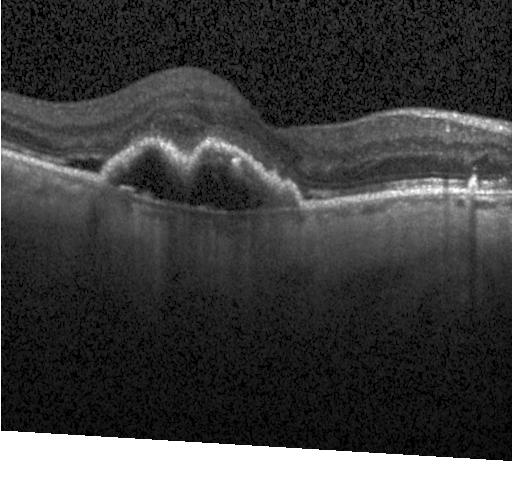

This B-scan demonstrates a choroidal neovascular membrane.